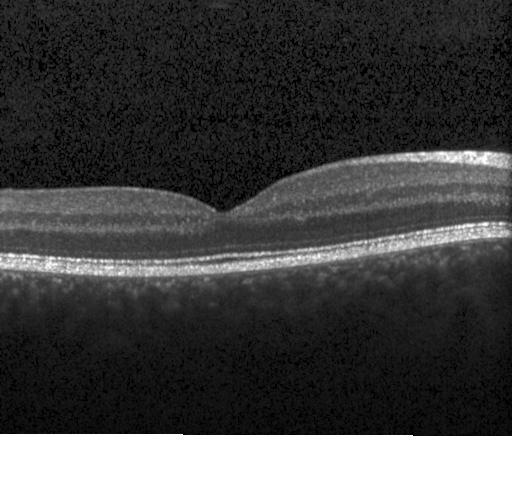 Spectral-domain OCT. Optical coherence tomography scan.
Macular OCT: no CNV, DME, or drusen.